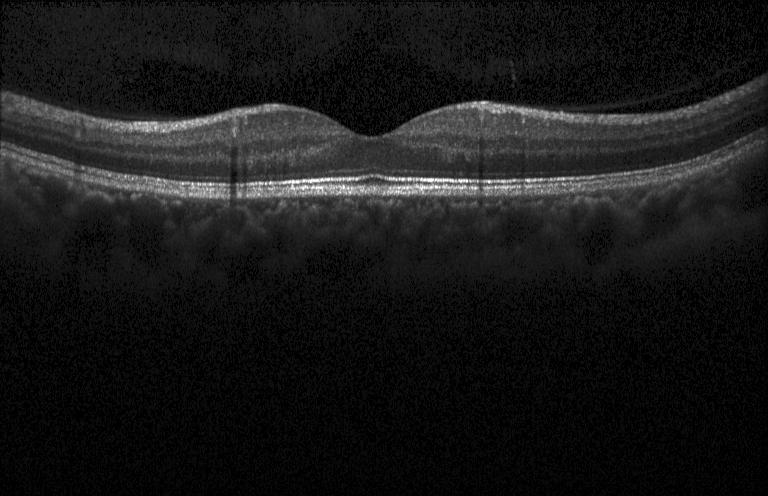
This B-scan demonstrates no CNV, no DME, and no drusen.